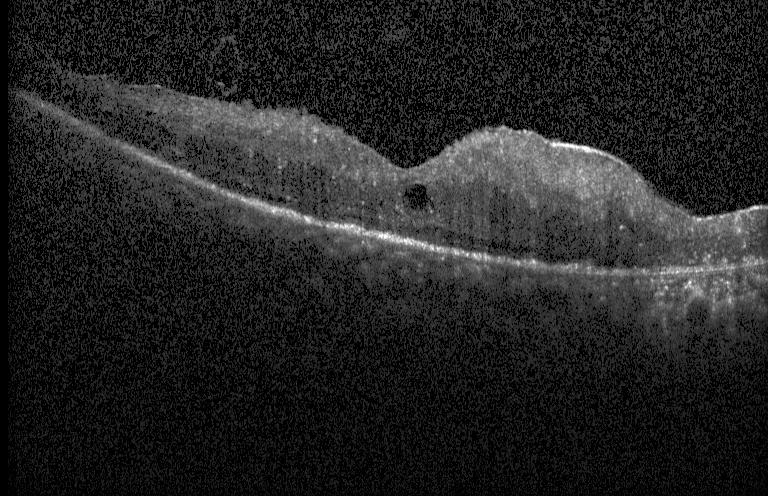

OCT B-scan showing diabetic macular edema.